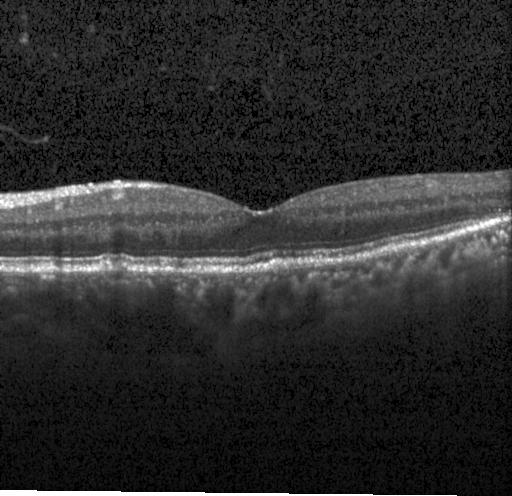

Heidelberg Spectralis OCT system, spectral-domain OCT, optical coherence tomography B-scan — Assessment: drusen.